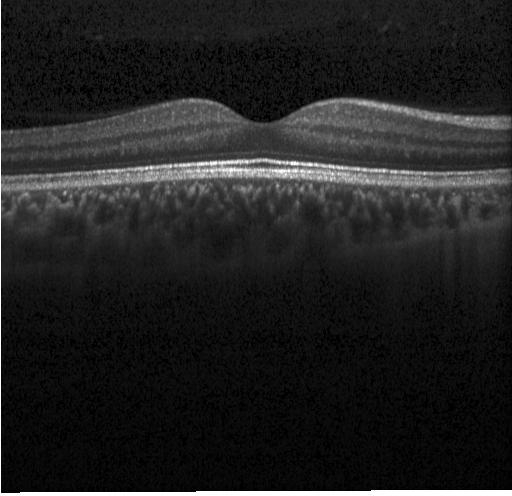 Diagnosis: neither choroidal neovascularization, diabetic macular edema, nor drusen.